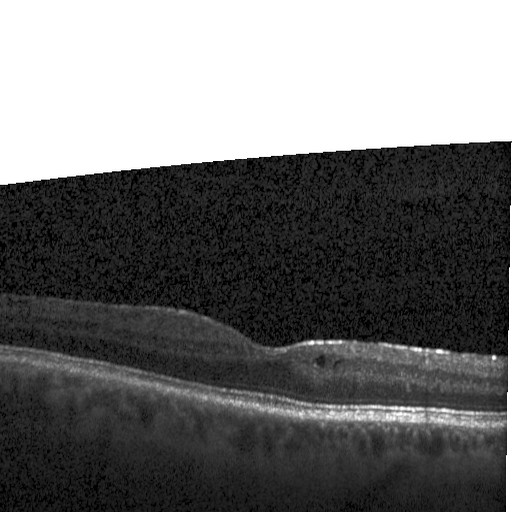

Macular OCT demonstrating DME.